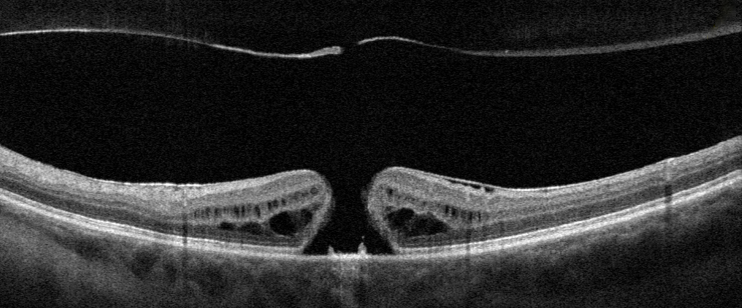

Finding: vitreomacular interface disease (VID).